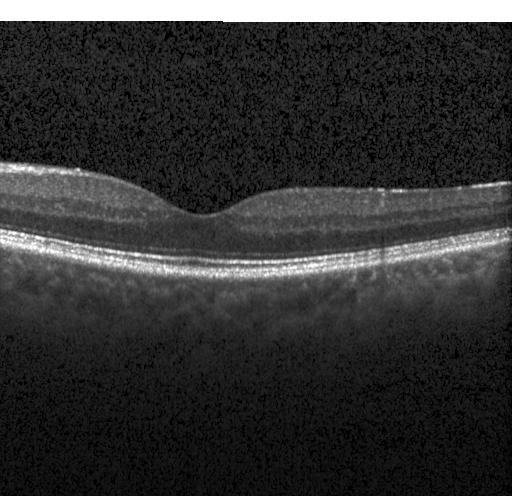
Horizontal scan through the fovea. Retinal OCT B-scan. Heidelberg Spectralis.
Diagnosis: no choroidal neovascularization, diabetic macular edema, or drusen.